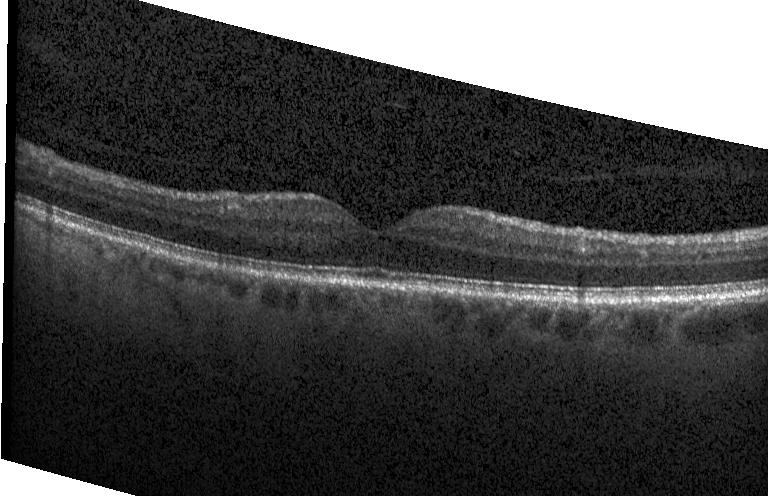 OCT B-scan showing no choroidal neovascularization, no diabetic macular edema, and no drusen.